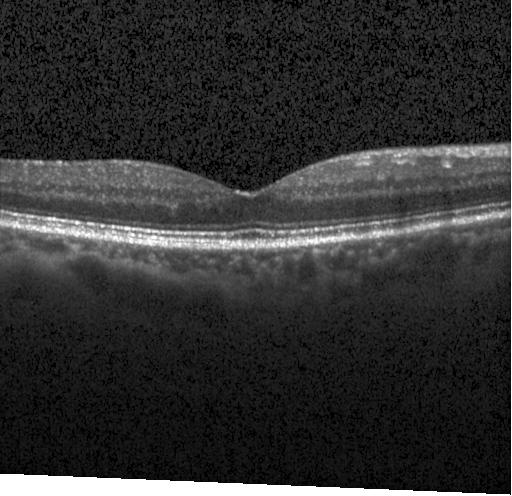

Optical coherence tomography scan — Assessment: no choroidal neovascularization, diabetic macular edema, or drusen.